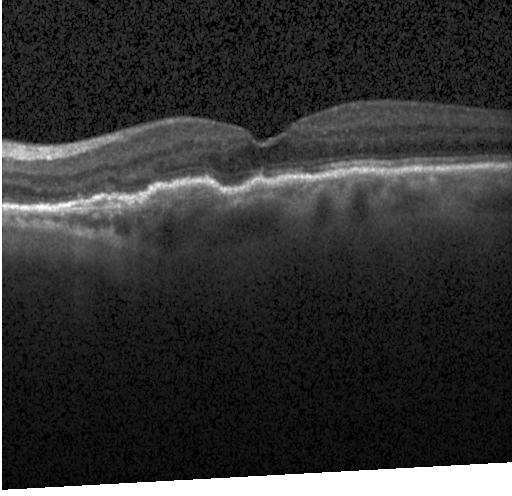

SD-OCT · OCT B-scan · Heidelberg Spectralis OCT system. Finding: a choroidal neovascular membrane.